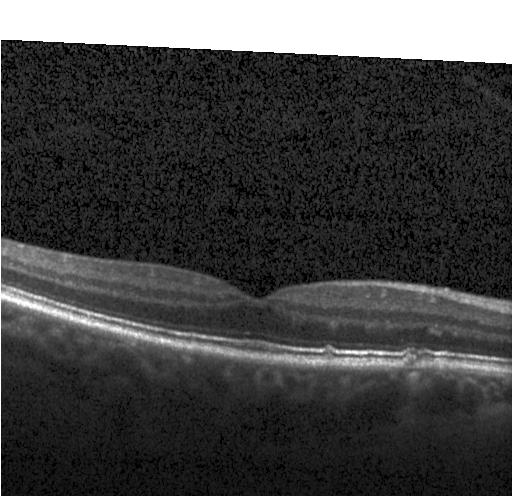

OCT B-scan; Heidelberg Spectralis OCT system; SD-OCT
Drusen.